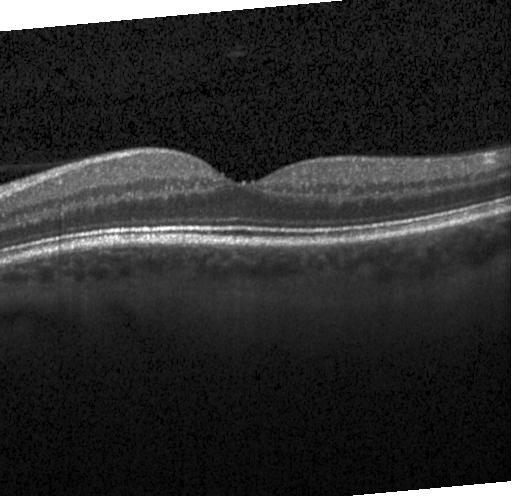

Optical coherence tomography B-scan, SD-OCT. Dx: no choroidal neovascularization, no diabetic macular edema, and no drusen.